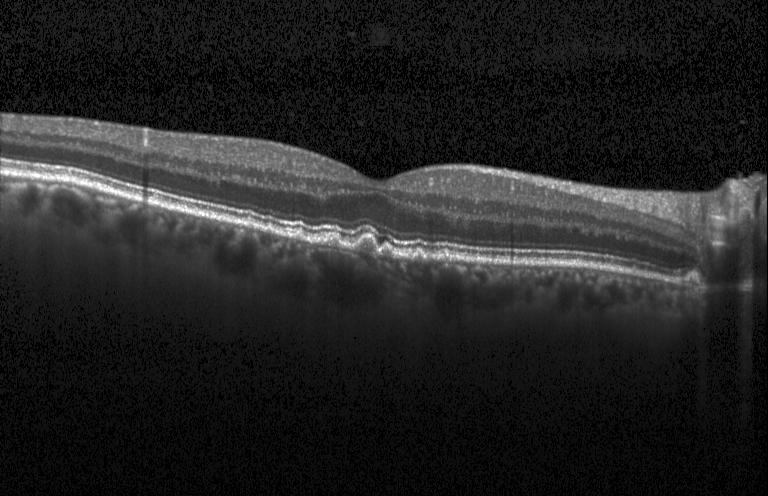

Spectral-domain optical coherence tomography · Heidelberg Spectralis · optical coherence tomography scan · centered on the fovea. Impression: multiple drusen.